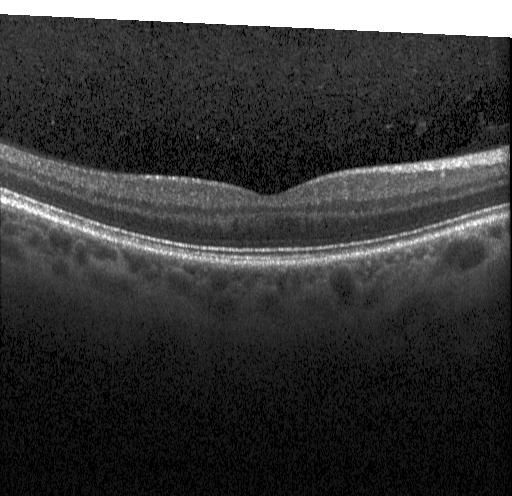
Retinal OCT B-scan, fovea-centered, SD-OCT, Heidelberg Spectralis. This B-scan demonstrates no evidence of choroidal neovascularization, diabetic macular edema, or drusen.